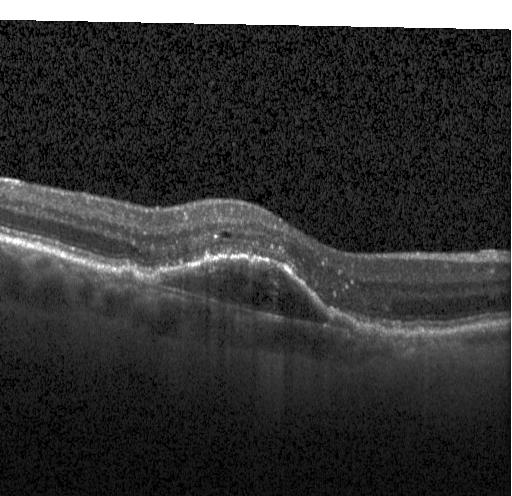 OCT B-scan. Macular OCT: a choroidal neovascular membrane.